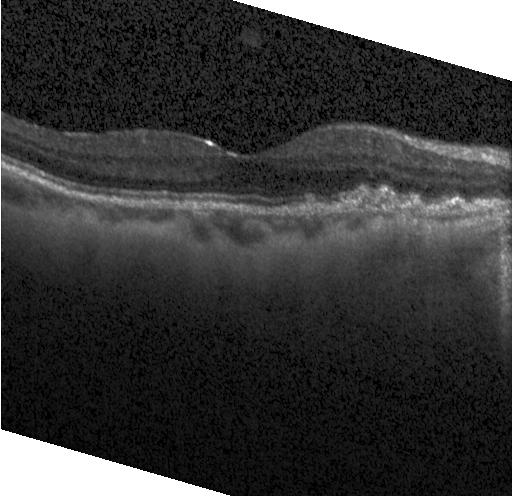 Optical coherence tomography scan.
Diagnosis: sub-RPE drusenoid deposits.